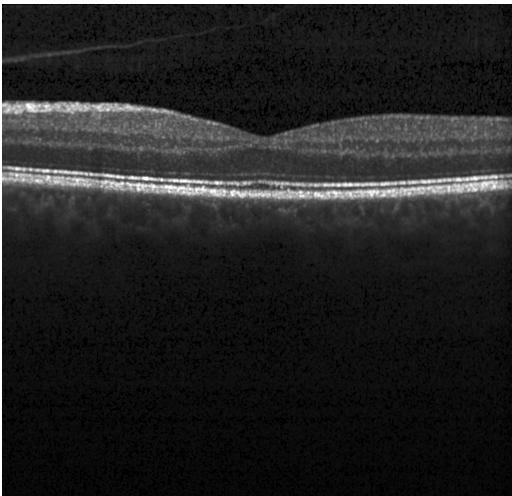
Acquired on a Heidelberg Spectralis, fovea-centered, OCT line scan — Impression: neither choroidal neovascularization, diabetic macular edema, nor drusen.